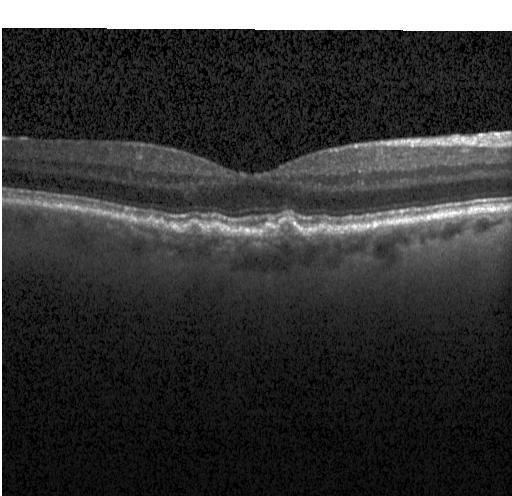

Dx: multiple drusen.